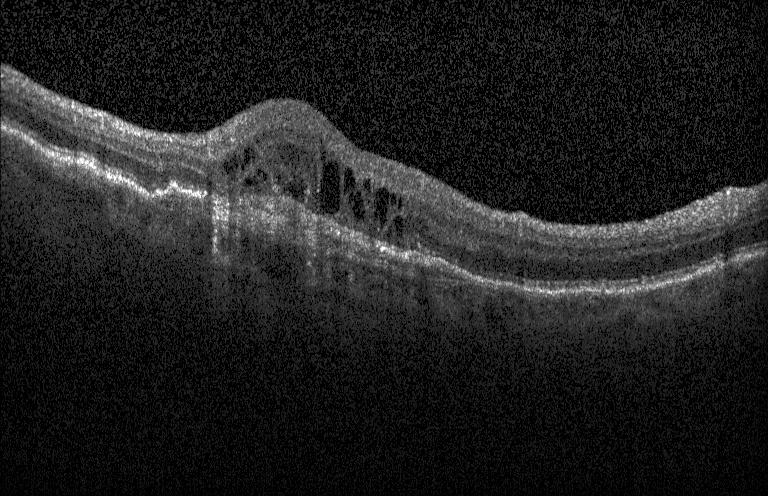

Retinal OCT B-scan, acquired on a Heidelberg Spectralis.
Assessment: a choroidal neovascular membrane.